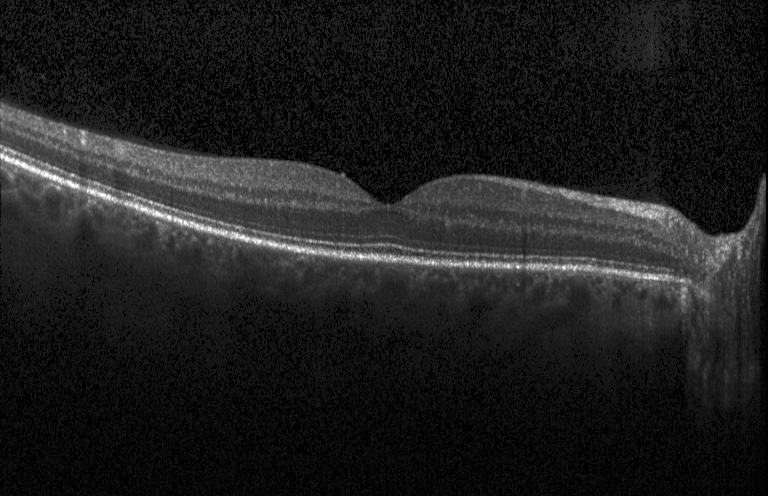

Acquired on a Heidelberg Spectralis. Optical coherence tomography B-scan. No CNV, DME, or drusen.